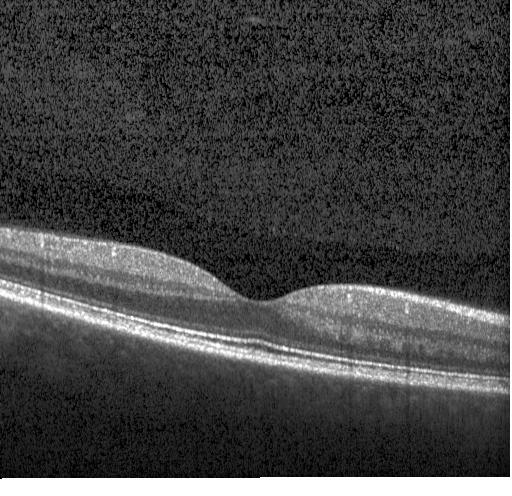

OCT B-scan — The scan shows no choroidal neovascularization, no diabetic macular edema, and no drusen.